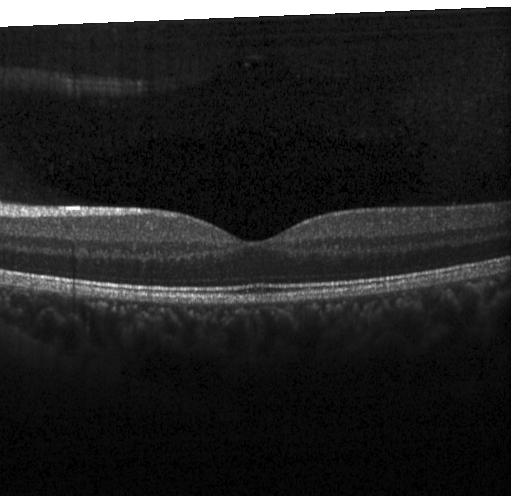

SD-OCT. OCT line scan. Heidelberg Spectralis OCT system. Fovea-centered. Finding: no evidence of CNV, DME, or drusen.